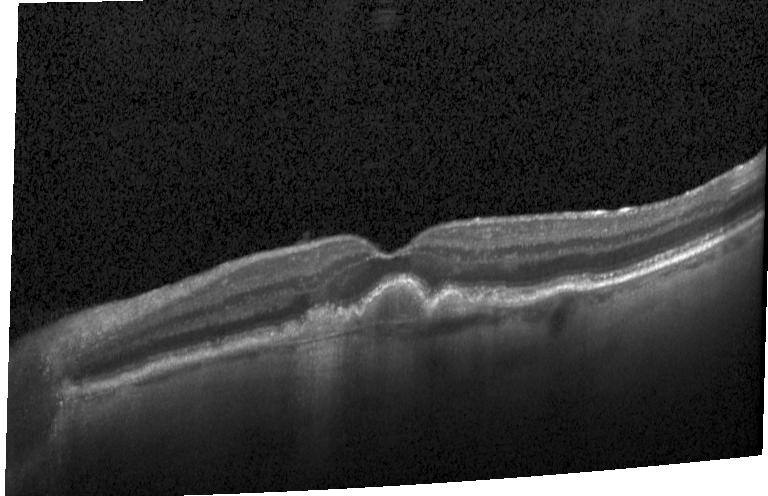

Diagnosis: a choroidal neovascular membrane.